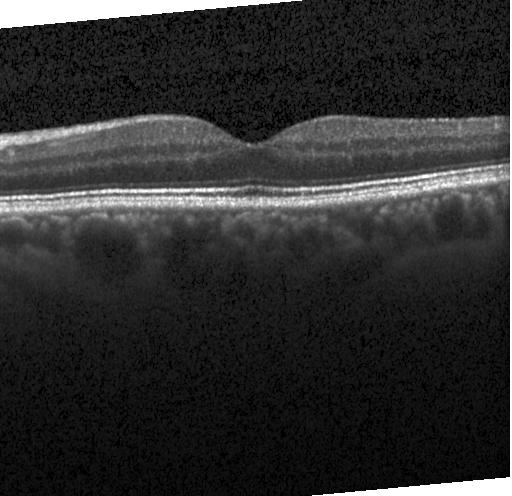 Instrument: Heidelberg Spectralis; optical coherence tomography scan; fovea-centered; spectral-domain optical coherence tomography.
This B-scan demonstrates no choroidal neovascularization, no diabetic macular edema, and no drusen.